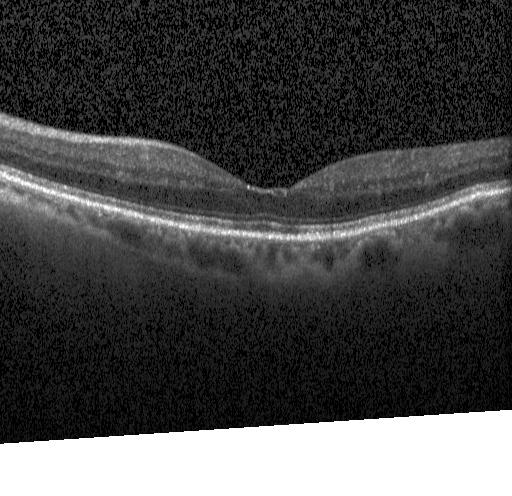 Optical coherence tomography scan — Assessment: no CNV, DME, or drusen.